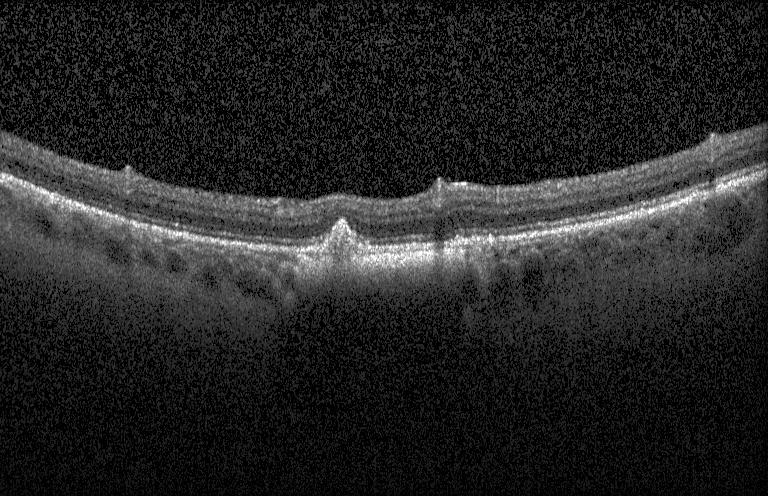
Retinal OCT B-scan · spectral-domain OCT · acquired on a Heidelberg Spectralis · through the macula — OCT finding: choroidal neovascularization (CNV).